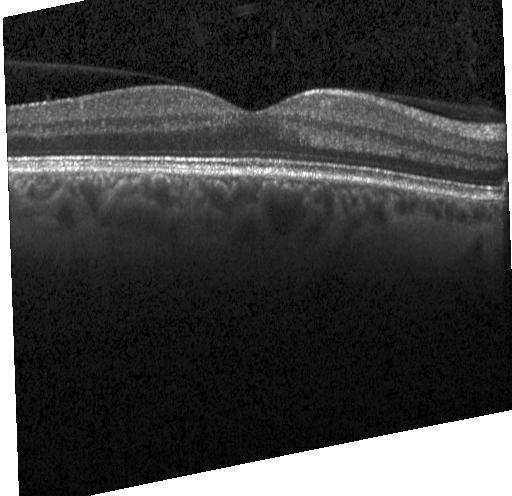
Instrument: Heidelberg Spectralis, OCT B-scan. Impression: no CNV, DME, or drusen.